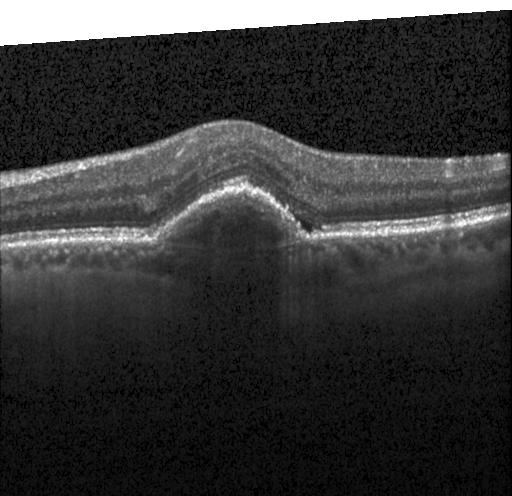 Impression: choroidal neovascularization.